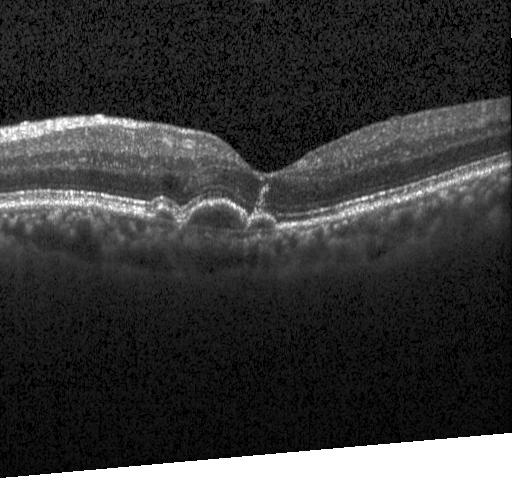

Instrument: Heidelberg Spectralis · fovea-centered · optical coherence tomography scan · SD-OCT — Assessment: a choroidal neovascular membrane.